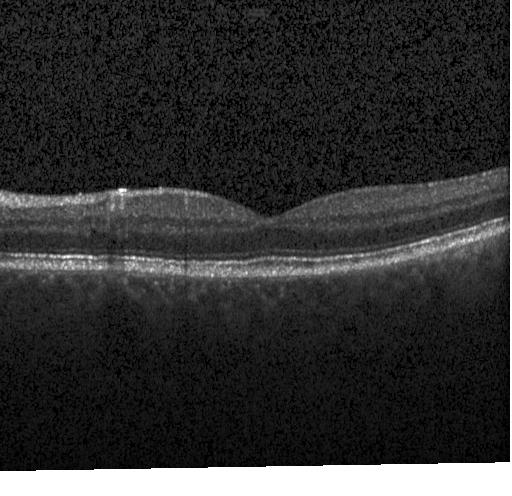
Diagnosis: no CNV, DME, or drusen.